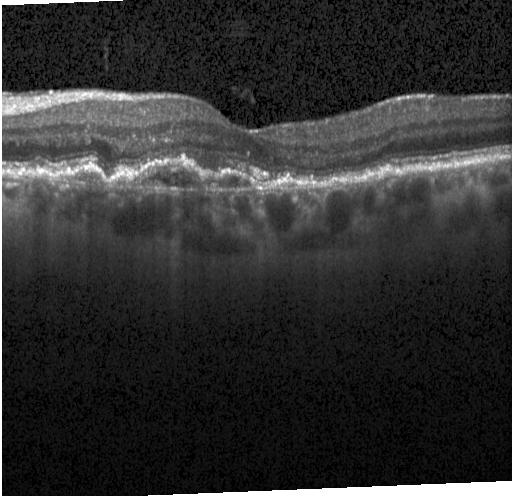 Retinal OCT cross-section. Spectral-domain OCT. Acquired on a Heidelberg Spectralis. Horizontal scan through the fovea — Macular OCT: CNV.